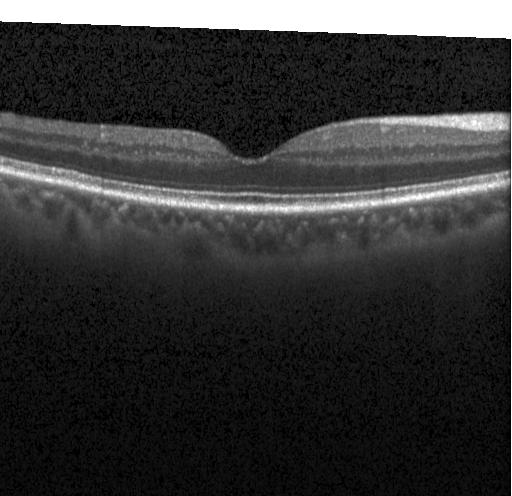
Spectral-domain OCT B-scan: no evidence of CNV, DME, or drusen.